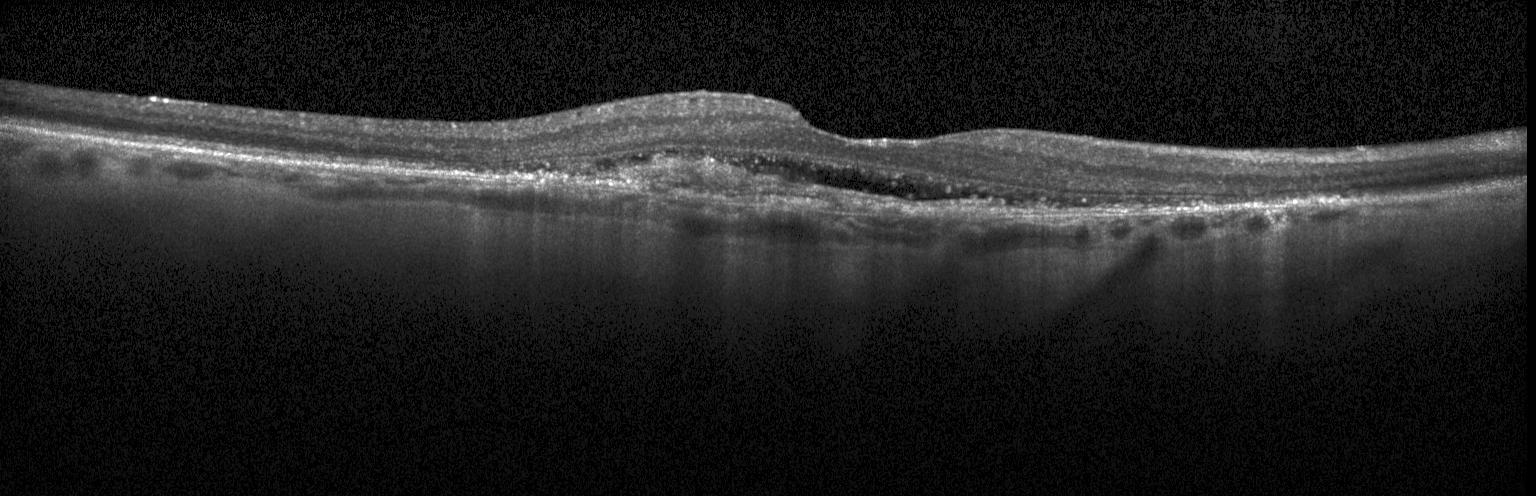 Optical coherence tomography scan, fovea-centered, acquired on a Heidelberg Spectralis — This B-scan demonstrates a choroidal neovascular membrane.